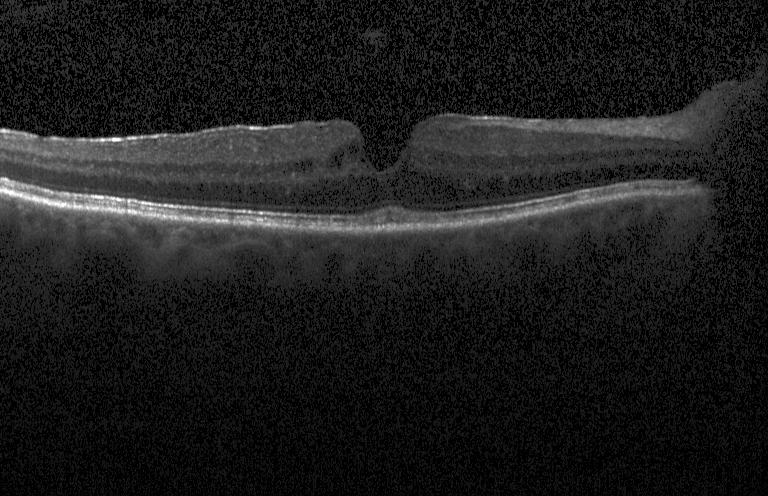

This B-scan demonstrates diabetic macular edema (DME).